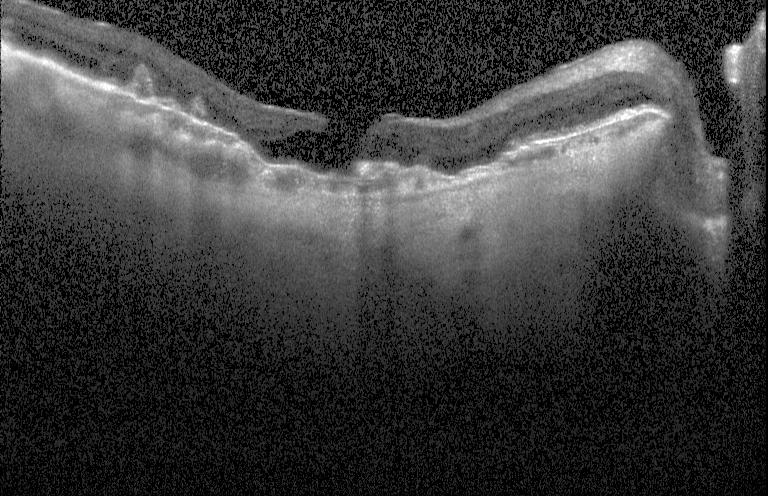
OCT line scan
Assessment: a choroidal neovascular membrane.